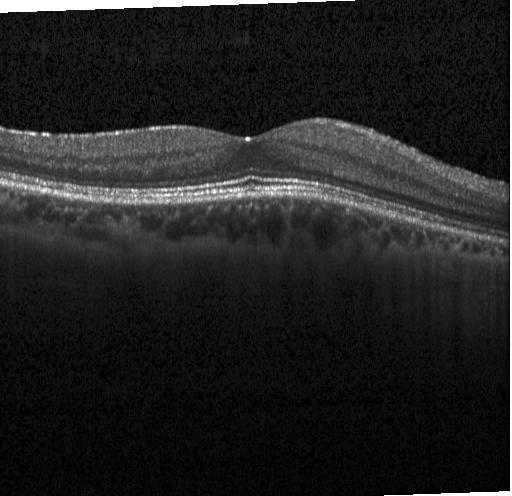 Impression: no evidence of choroidal neovascularization, diabetic macular edema, or drusen.